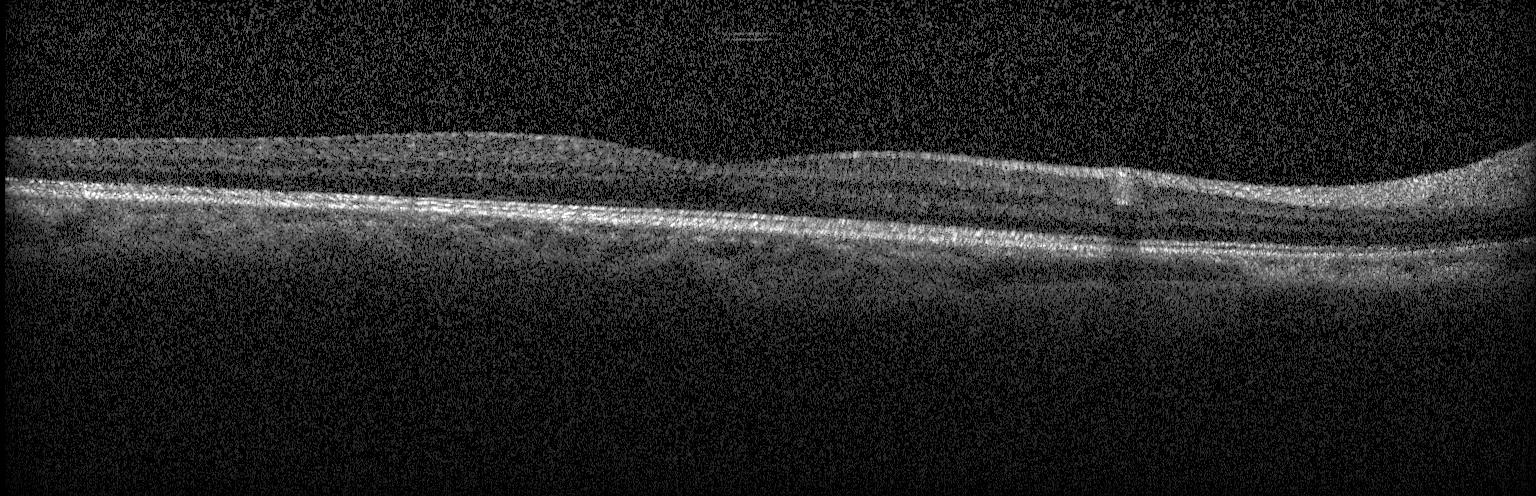

Acquired on a Heidelberg Spectralis; optical coherence tomography scan. Finding: no evidence of CNV, DME, or drusen.